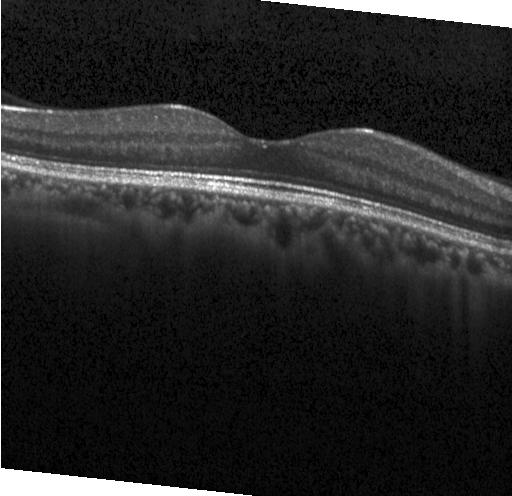 SD-OCT; optical coherence tomography B-scan; fovea-centered. Impression: neither choroidal neovascularization, diabetic macular edema, nor drusen.